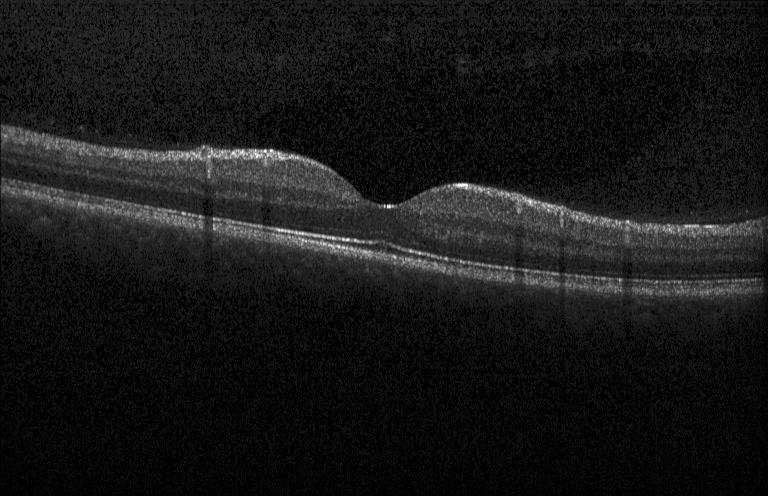
Impression: no evidence of choroidal neovascularization, diabetic macular edema, or drusen.